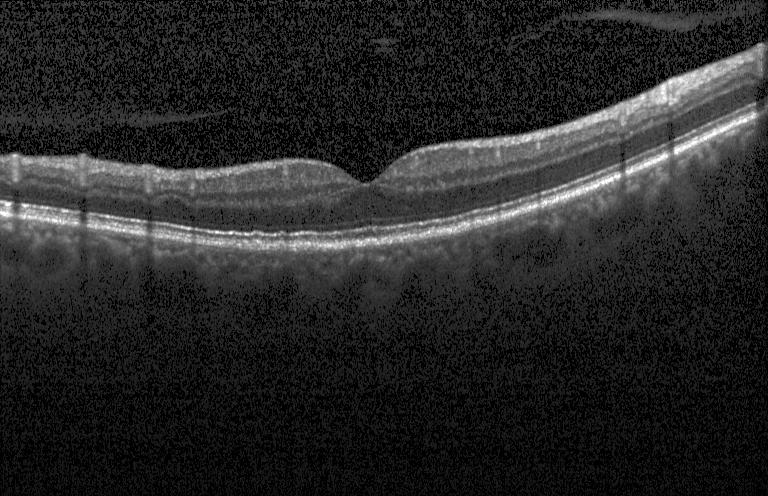

Finding: neither choroidal neovascularization, diabetic macular edema, nor drusen.